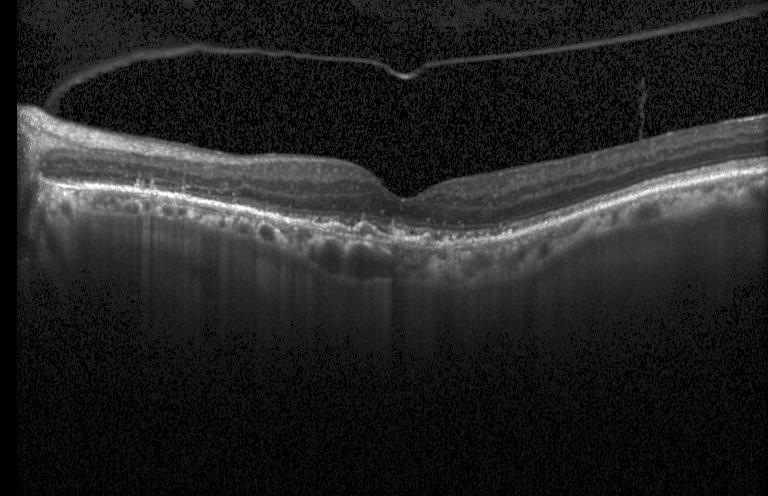

Diagnosis: a choroidal neovascular membrane.